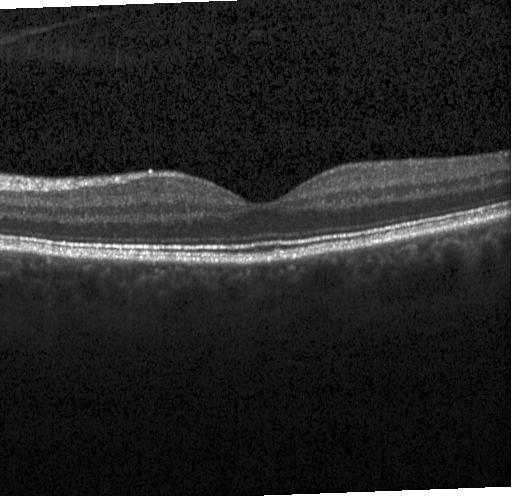
SD-OCT; retinal OCT cross-section
Assessment: no evidence of choroidal neovascularization, diabetic macular edema, or drusen.